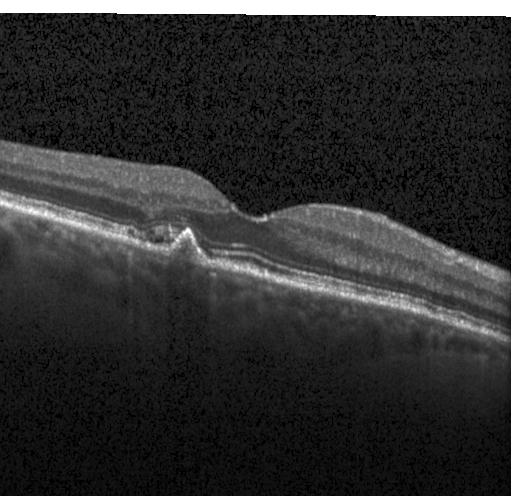 Macular scan; spectral-domain optical coherence tomography; retinal OCT cross-section.
Finding: a choroidal neovascular membrane.